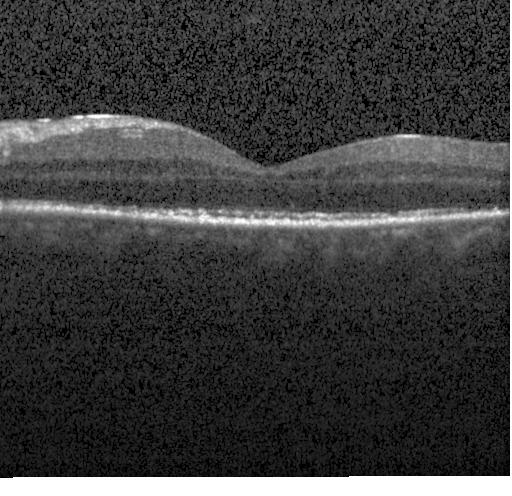
Retinal OCT B-scan. The scan shows no CNV, no DME, and no drusen.